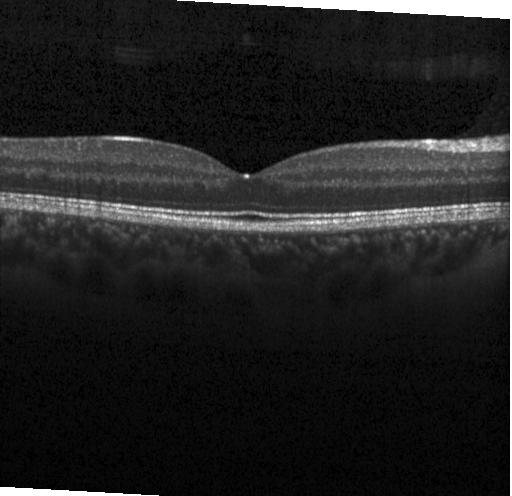 Centered on the fovea. Heidelberg Spectralis. Optical coherence tomography B-scan. SD-OCT.
Finding: no choroidal neovascularization, no diabetic macular edema, and no drusen.